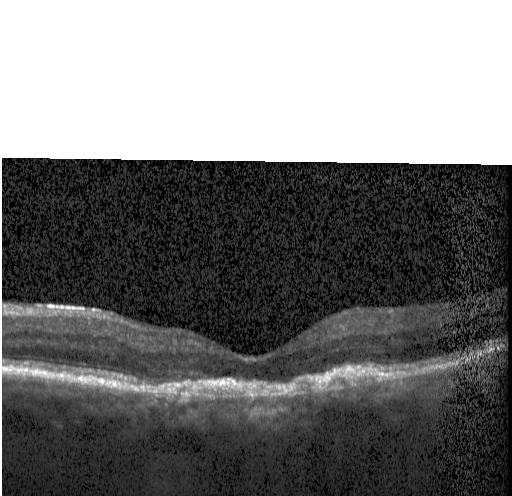 Optical coherence tomography B-scan
Impression: a choroidal neovascular membrane.